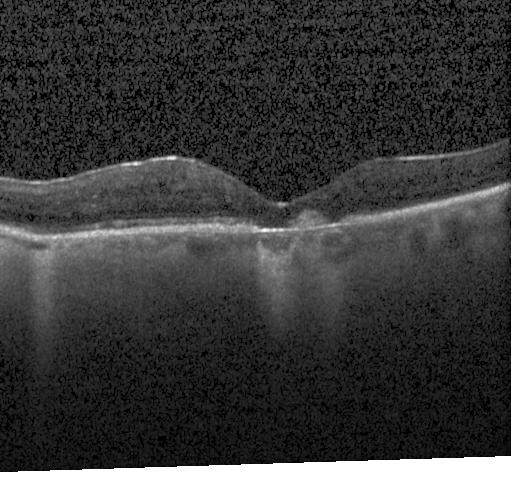
OCT scan showing choroidal neovascularization.